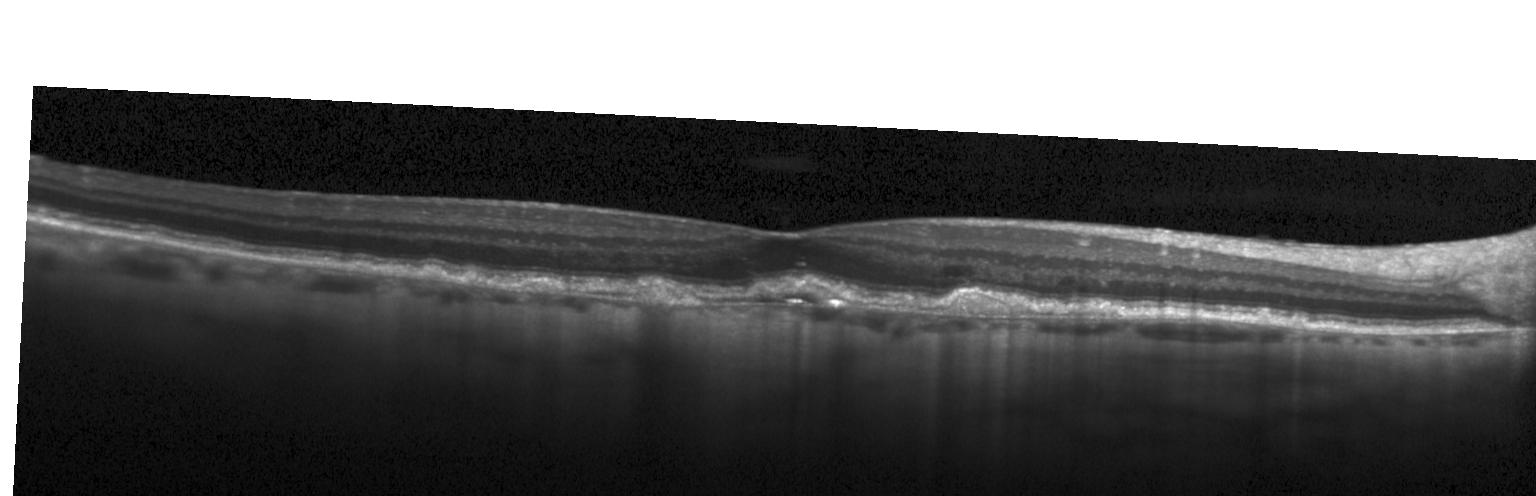
Macular OCT demonstrating choroidal neovascularization.